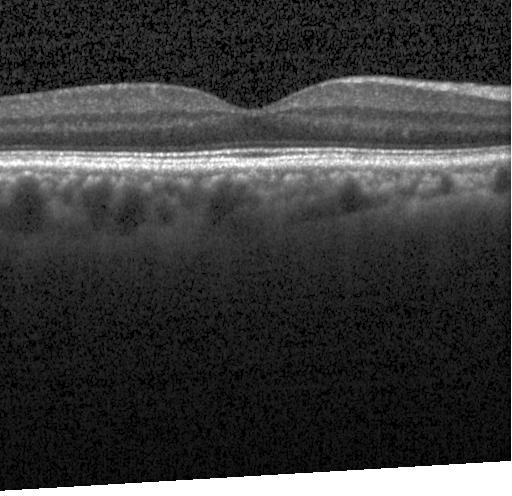

This B-scan demonstrates neither CNV, DME, nor drusen.